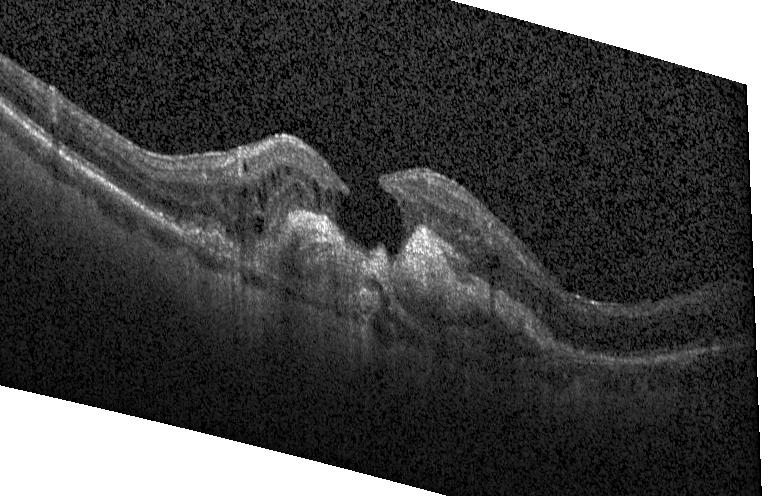

OCT scan showing CNV.